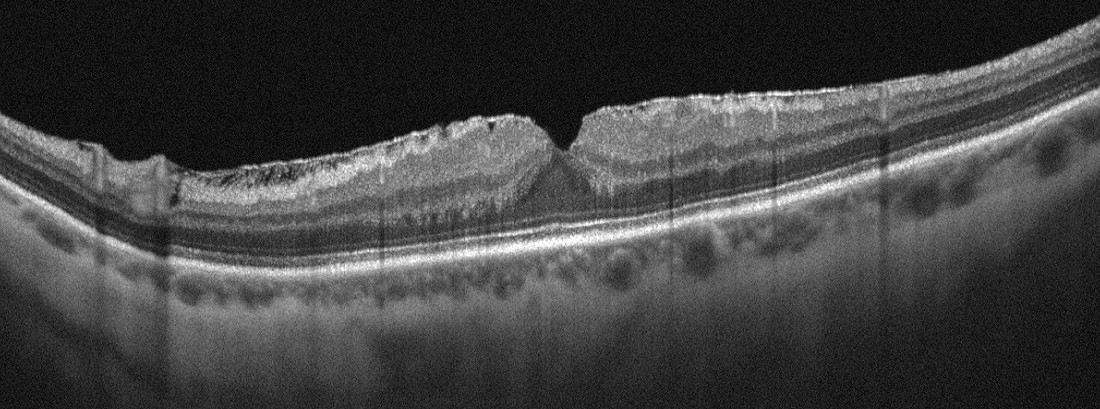 Retinal OCT B-scan.
Diagnosis: epiretinal membrane.